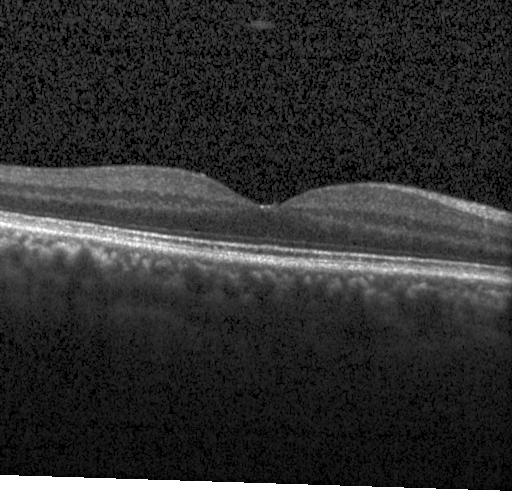
Acquired on a Heidelberg Spectralis; retinal OCT B-scan; SD-OCT; horizontal scan through the fovea
Dx: no evidence of choroidal neovascularization, diabetic macular edema, or drusen.